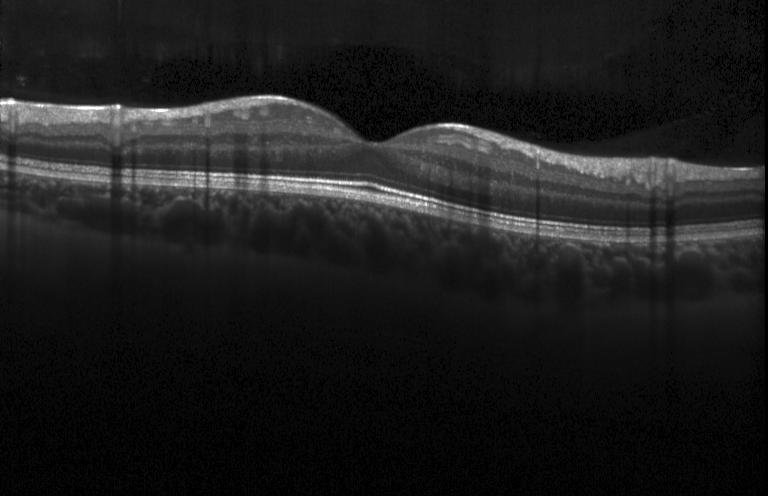 Macular OCT demonstrating no evidence of CNV, DME, or drusen.